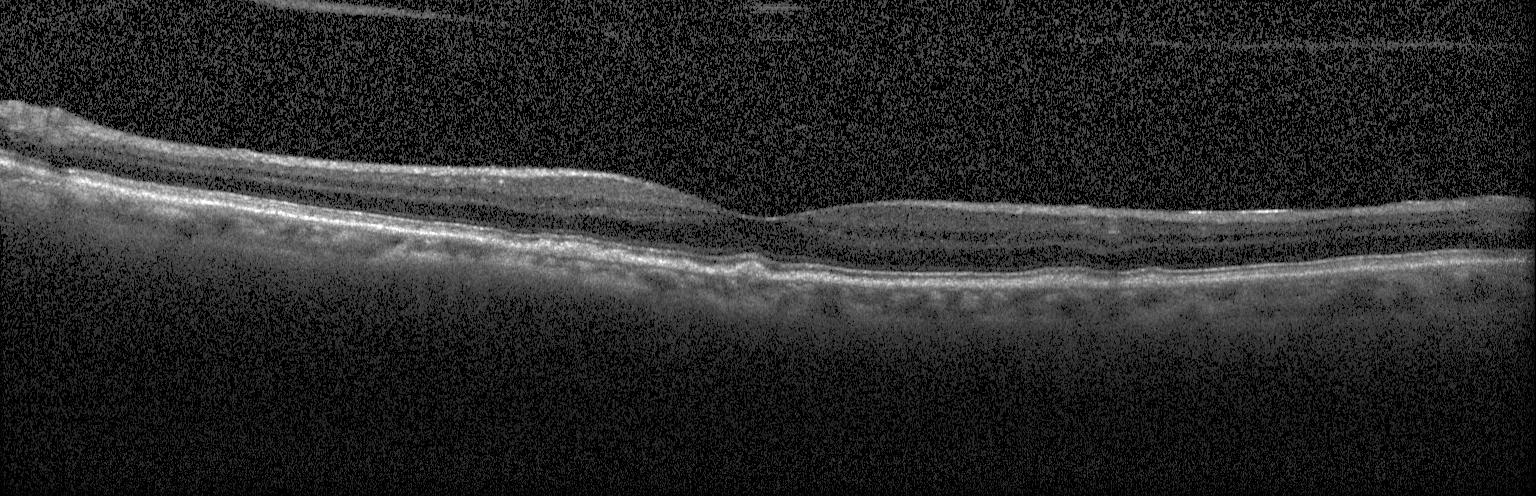 Centered on the fovea. Retinal OCT cross-section. SD-OCT.
Multiple drusen.